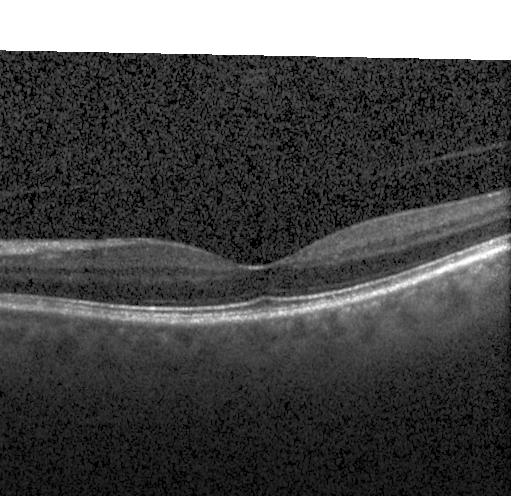 Finding: no evidence of choroidal neovascularization, diabetic macular edema, or drusen.